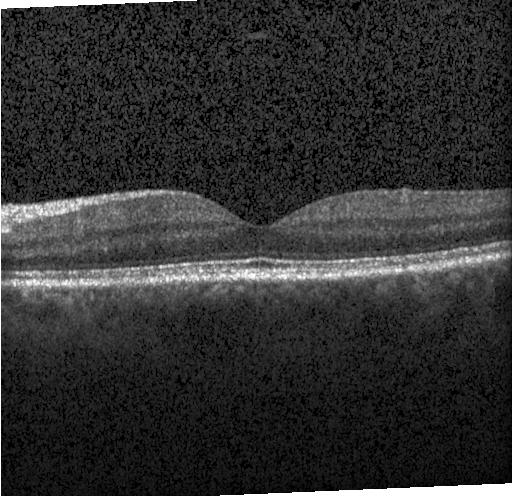

Instrument: Heidelberg Spectralis, centered on the fovea, SD-OCT, optical coherence tomography B-scan — Impression: no choroidal neovascularization, diabetic macular edema, or drusen.